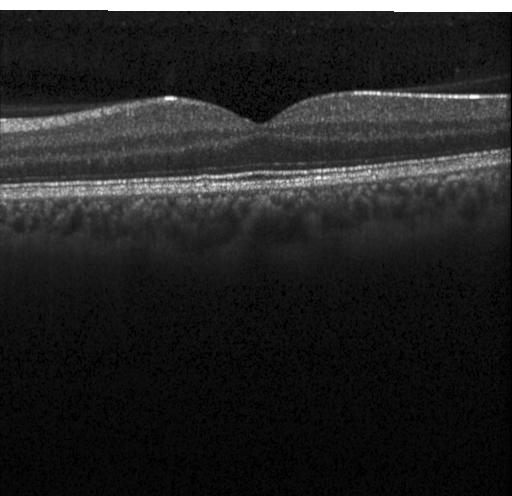

OCT finding: no evidence of choroidal neovascularization, diabetic macular edema, or drusen.